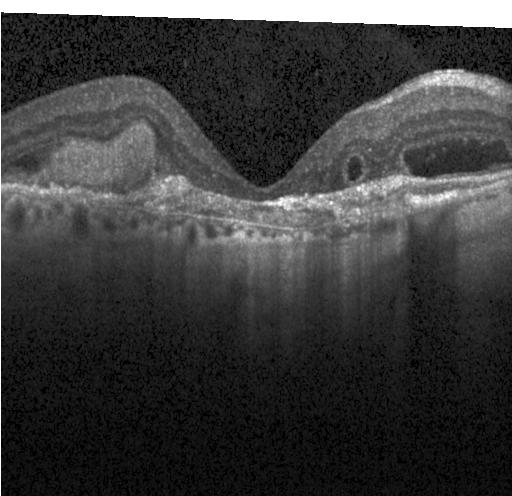 Retinal OCT cross-section showing a choroidal neovascular membrane.